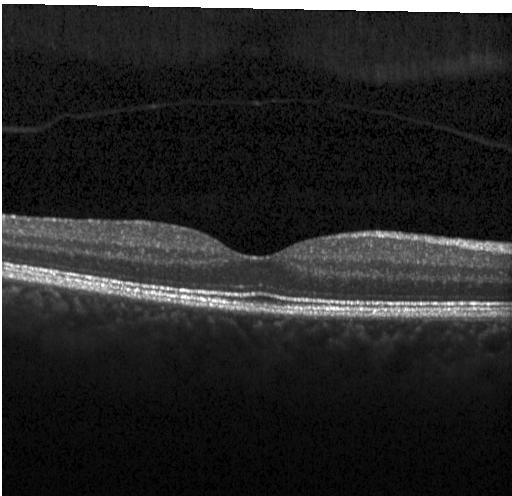

Retinal OCT B-scan · horizontal scan through the fovea
Impression: no evidence of choroidal neovascularization, diabetic macular edema, or drusen.